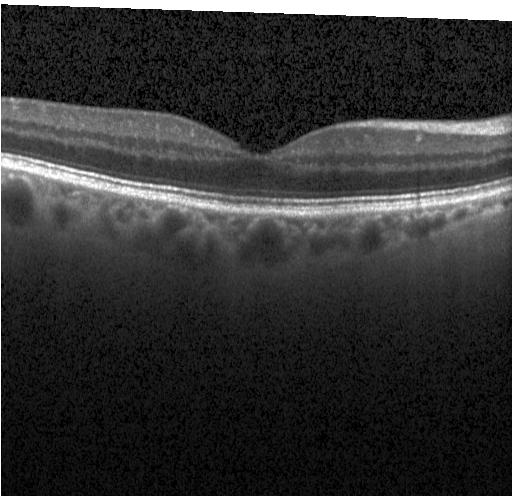 Optical coherence tomography scan.
Finding: no choroidal neovascularization, diabetic macular edema, or drusen.